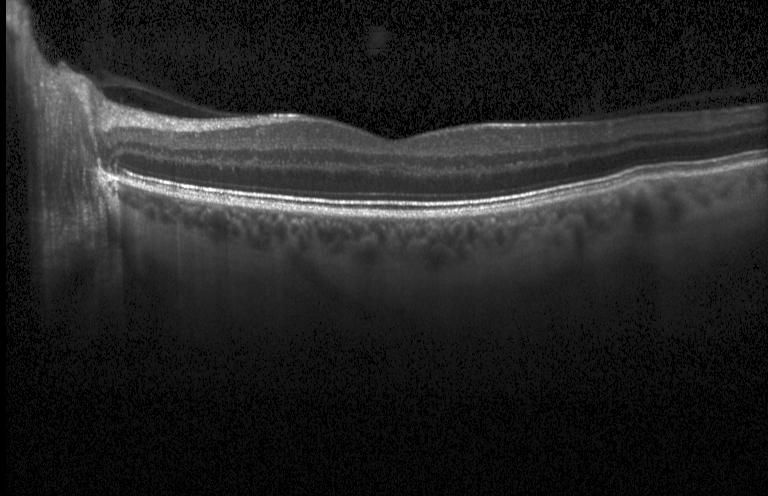
Impression: no evidence of choroidal neovascularization, diabetic macular edema, or drusen.